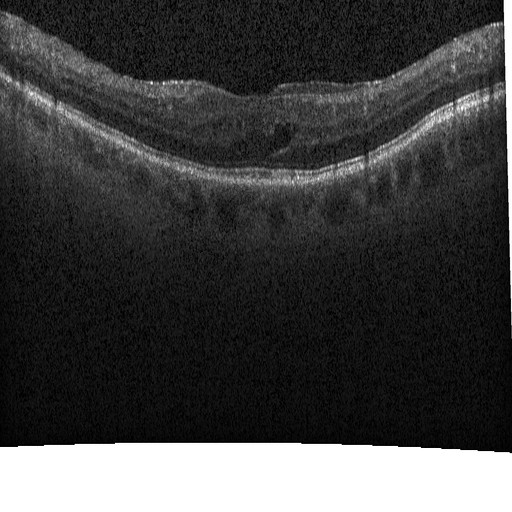
Spectral-domain OCT. OCT line scan. Macular scan.
Finding: diabetic macular edema (DME).